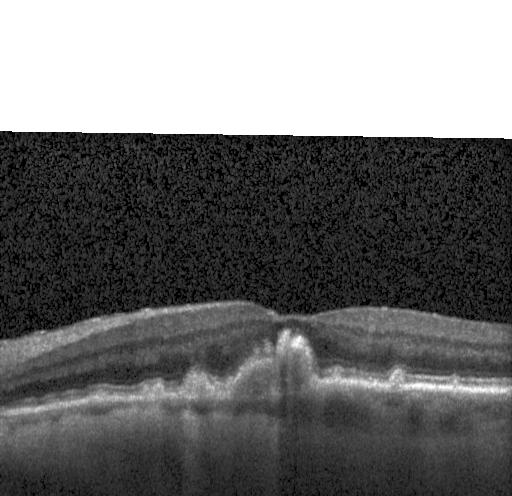
Acquired on a Heidelberg Spectralis. Optical coherence tomography B-scan. Macular scan — Impression: choroidal neovascularization (CNV).